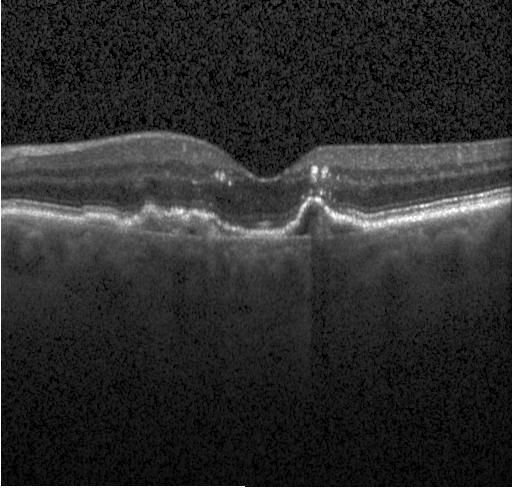
Instrument: Heidelberg Spectralis. Spectral-domain optical coherence tomography. Optical coherence tomography B-scan. Centered on the fovea
Diagnosis: choroidal neovascularization (CNV).